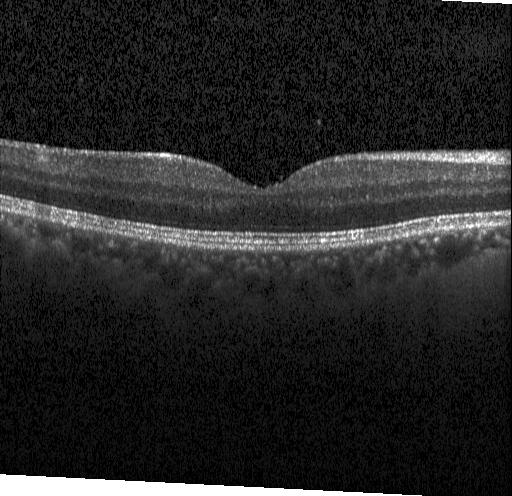 OCT line scan. Spectral-domain optical coherence tomography. Horizontal scan through the fovea. Finding: no evidence of choroidal neovascularization, diabetic macular edema, or drusen.